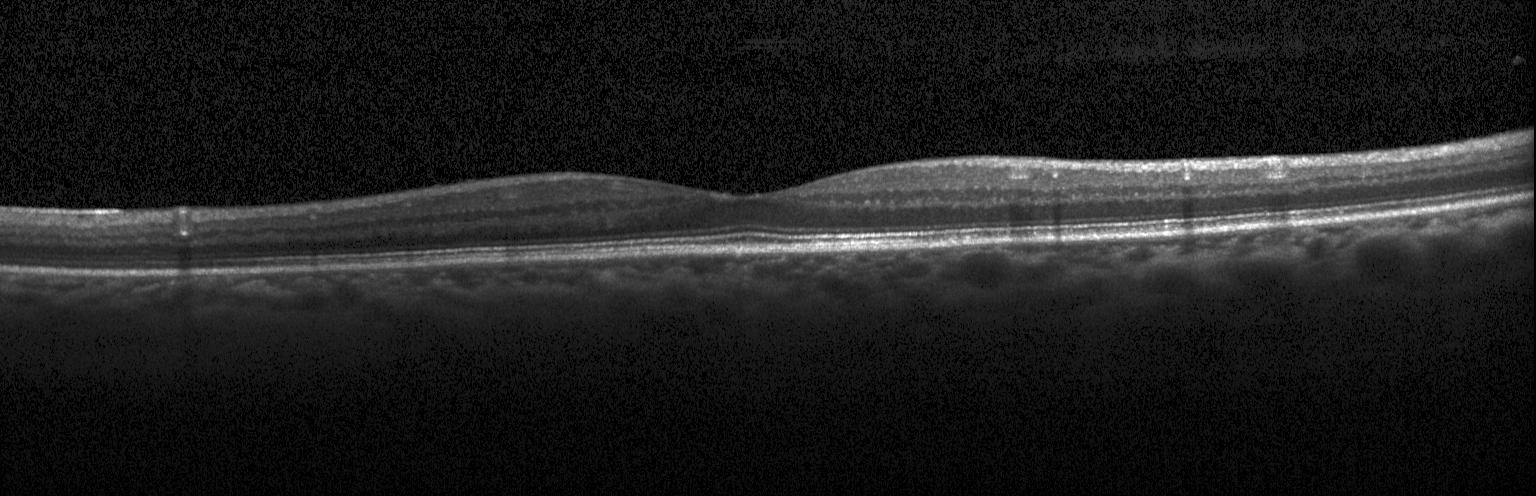

Optical coherence tomography B-scan
The scan shows no evidence of CNV, DME, or drusen.